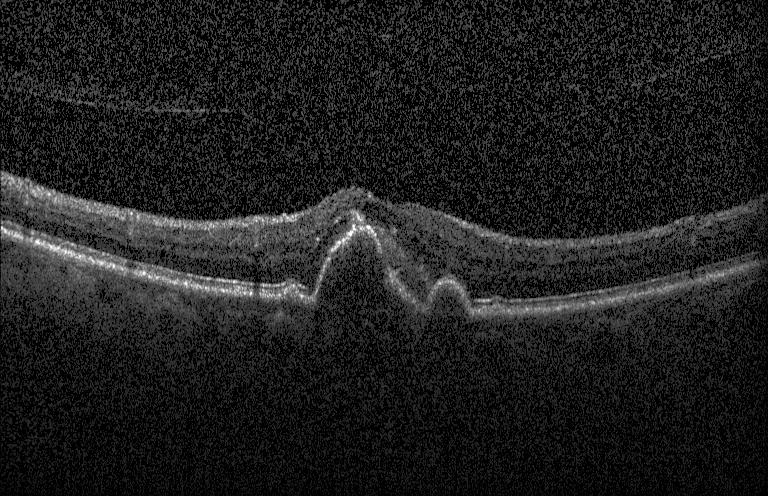 SD-OCT; Heidelberg Spectralis; retinal OCT cross-section; horizontal scan through the fovea — Impression: a choroidal neovascular membrane.